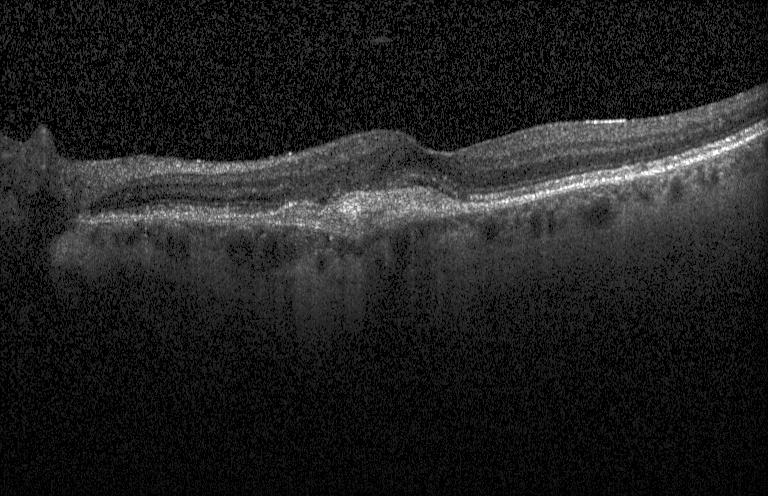
Retinal OCT B-scan.
Choroidal neovascularization.